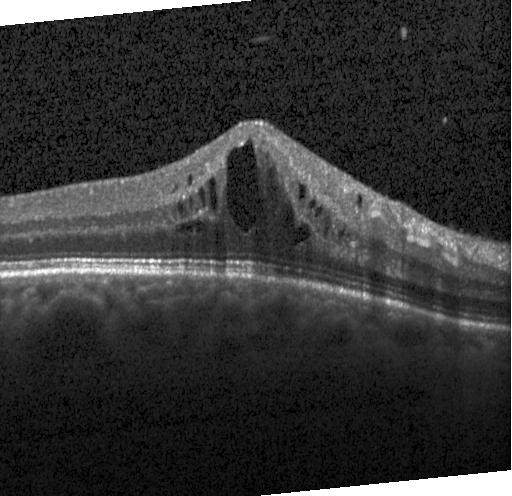

Fovea-centered, spectral-domain optical coherence tomography, OCT line scan.
Assessment: diabetic macular edema.